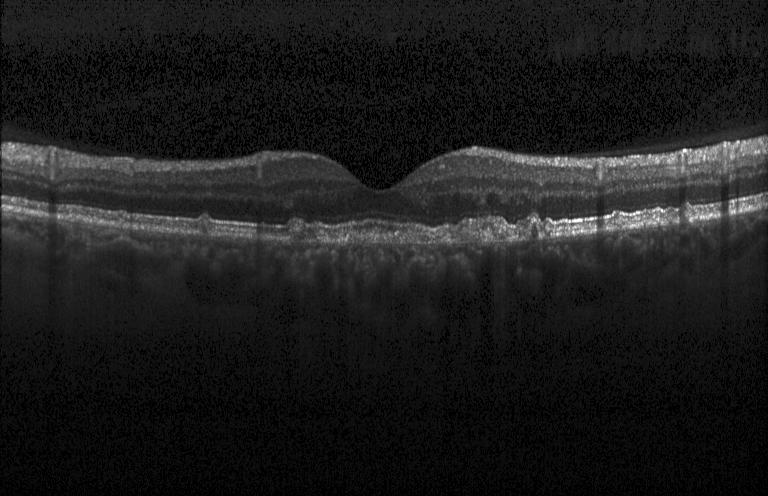
Impression: multiple drusen.